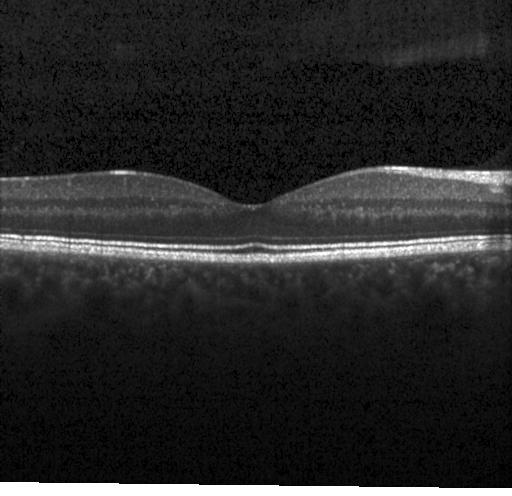

Macular OCT: no evidence of choroidal neovascularization, diabetic macular edema, or drusen.